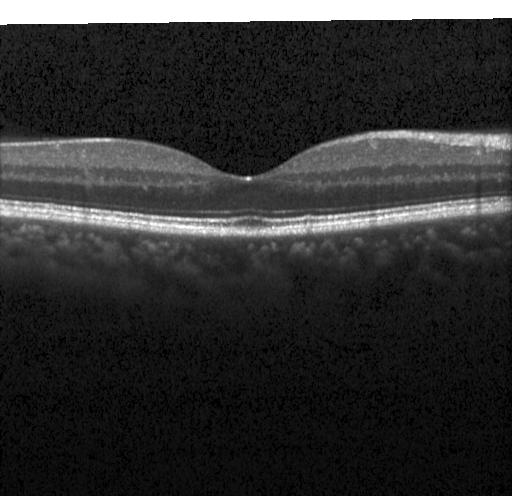
Optical coherence tomography scan — Diagnosis: neither choroidal neovascularization, diabetic macular edema, nor drusen.